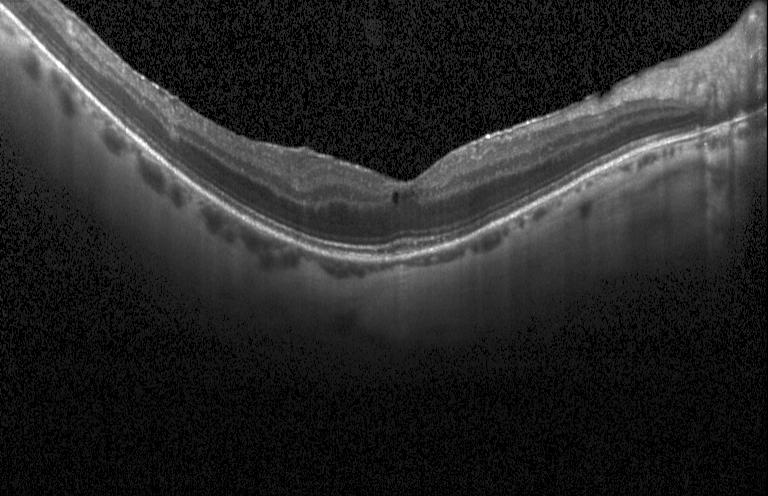 Optical coherence tomography B-scan, spectral-domain OCT. The scan shows DME.